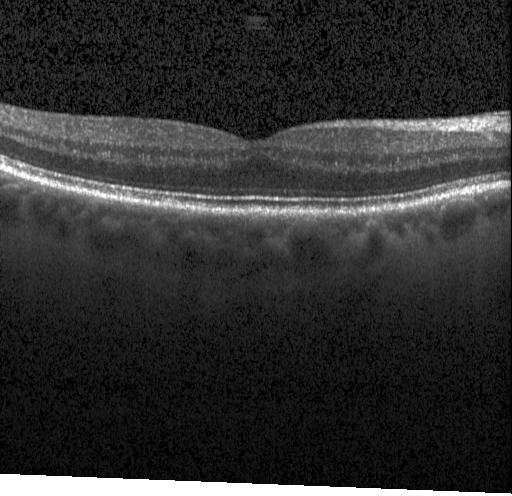
Macular OCT: no choroidal neovascularization, no diabetic macular edema, and no drusen.